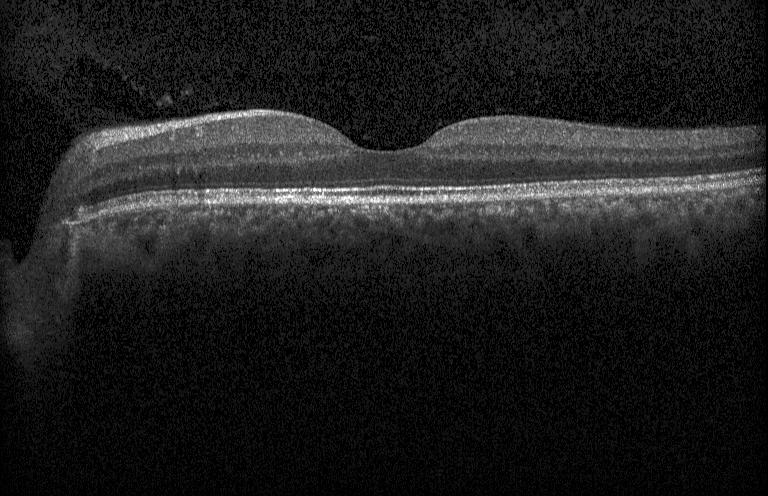
Retinal OCT cross-section, spectral-domain optical coherence tomography, Heidelberg Spectralis — Diagnosis: no evidence of choroidal neovascularization, diabetic macular edema, or drusen.